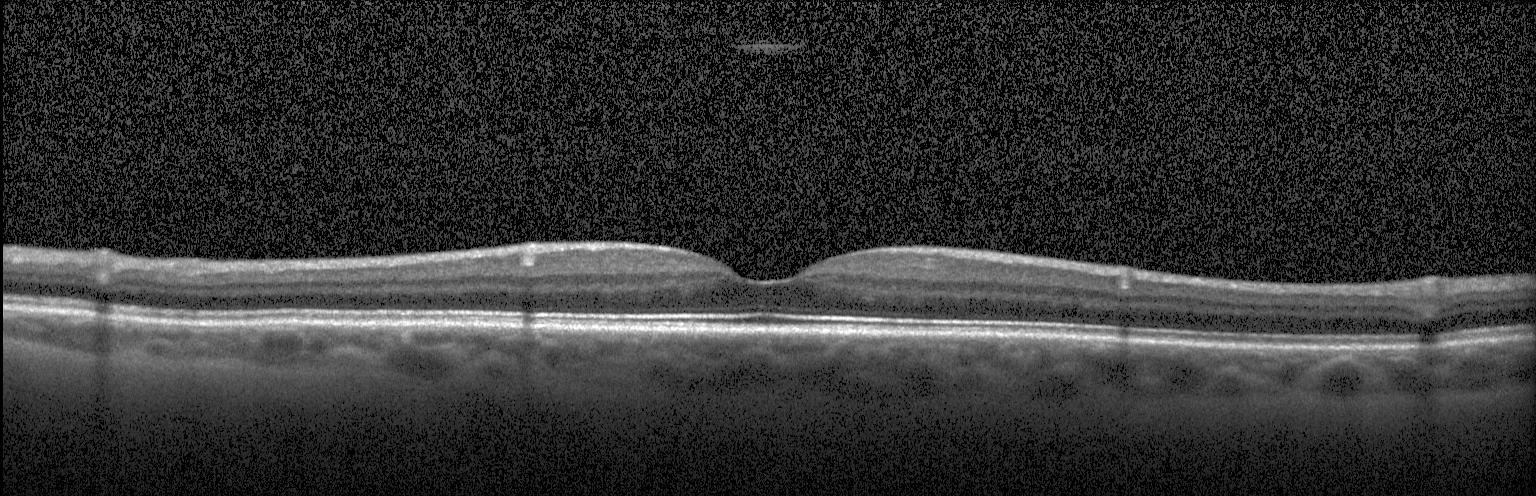
Retinal OCT cross-section
Impression: no choroidal neovascularization, no diabetic macular edema, and no drusen.